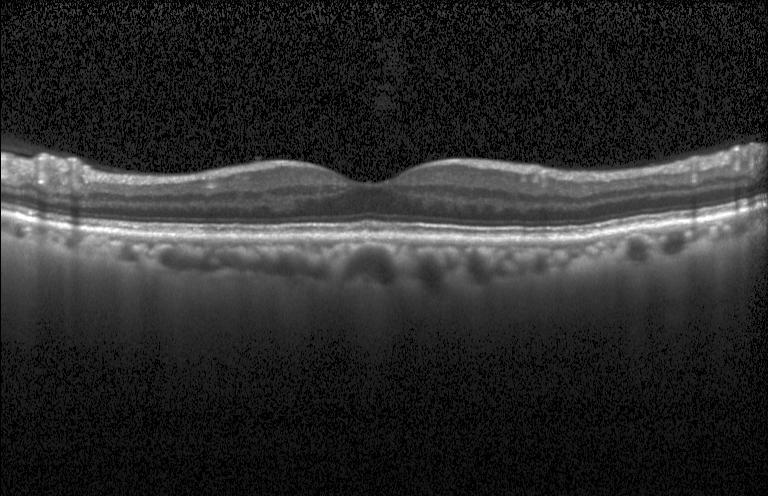
Heidelberg Spectralis OCT system, spectral-domain OCT, fovea-centered, OCT B-scan.
Finding: no CNV, DME, or drusen.